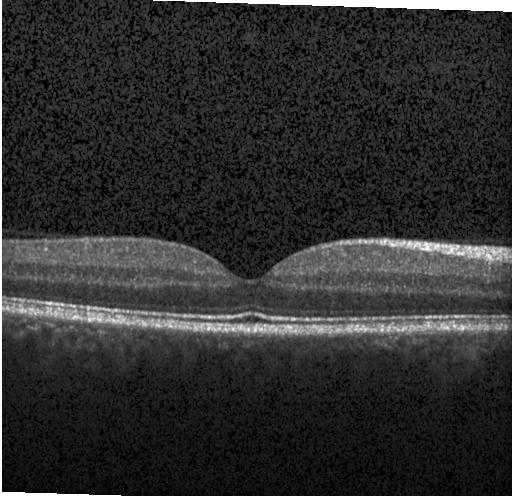 Optical coherence tomography B-scan, spectral-domain OCT. Finding: no evidence of choroidal neovascularization, diabetic macular edema, or drusen.